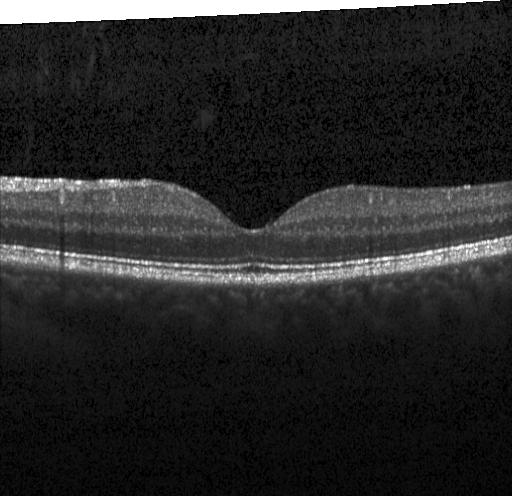 Spectral-domain OCT B-scan: no evidence of CNV, DME, or drusen.